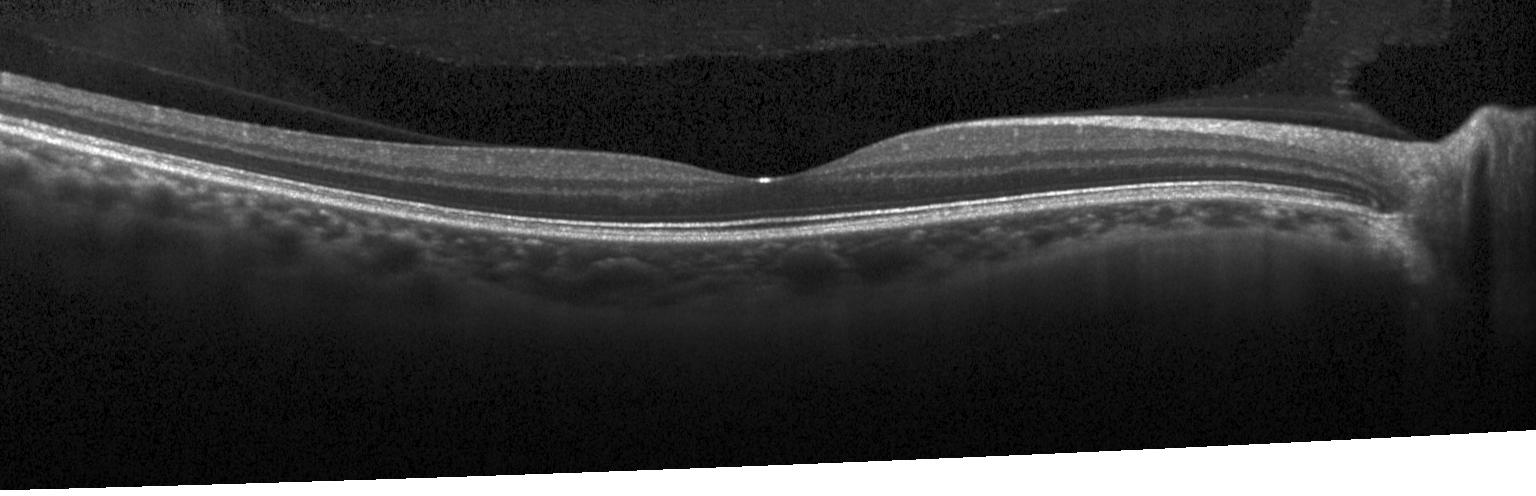

SD-OCT; through the macula; optical coherence tomography scan.
Impression: no choroidal neovascularization, diabetic macular edema, or drusen.